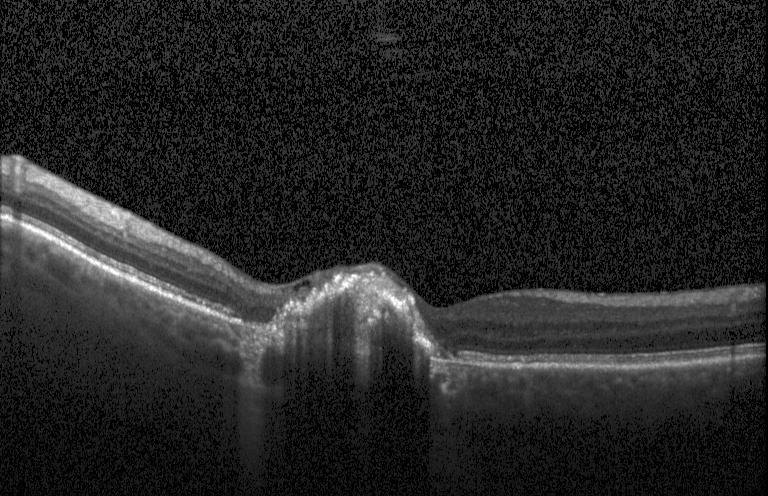 Finding: choroidal neovascularization.